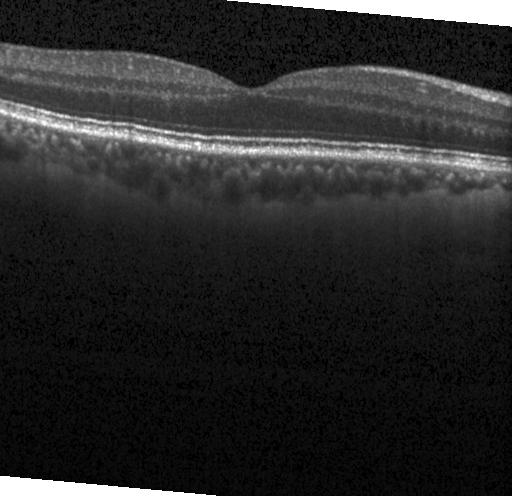 Centered on the fovea; OCT B-scan. Macular OCT: neither choroidal neovascularization, diabetic macular edema, nor drusen.